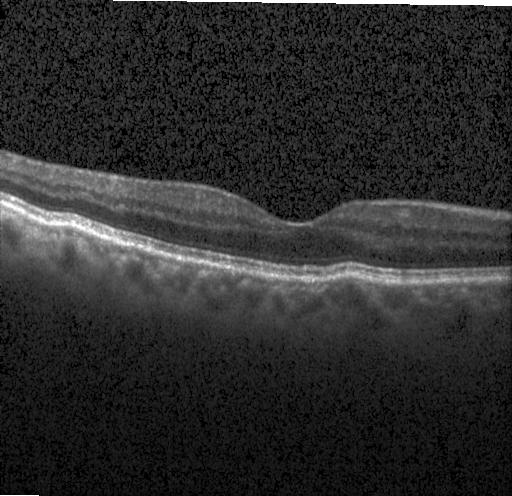 Retinal OCT B-scan; SD-OCT — The scan shows no choroidal neovascularization, diabetic macular edema, or drusen.